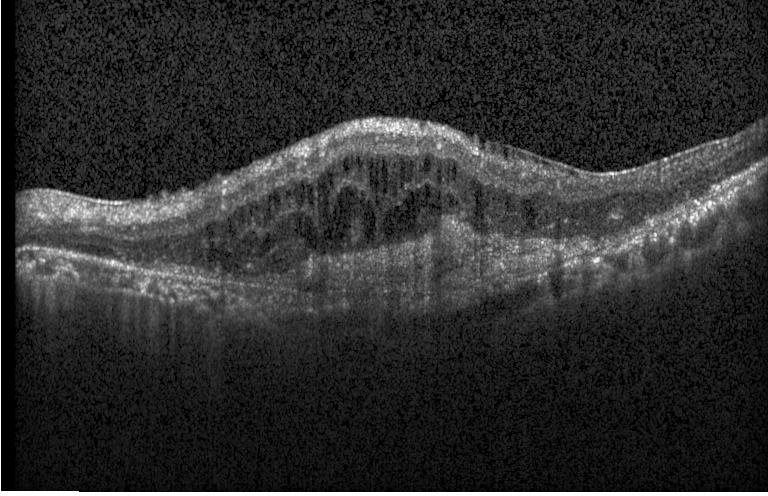
Optical coherence tomography B-scan · Heidelberg Spectralis OCT system · centered on the fovea · spectral-domain optical coherence tomography — Macular OCT: CNV.